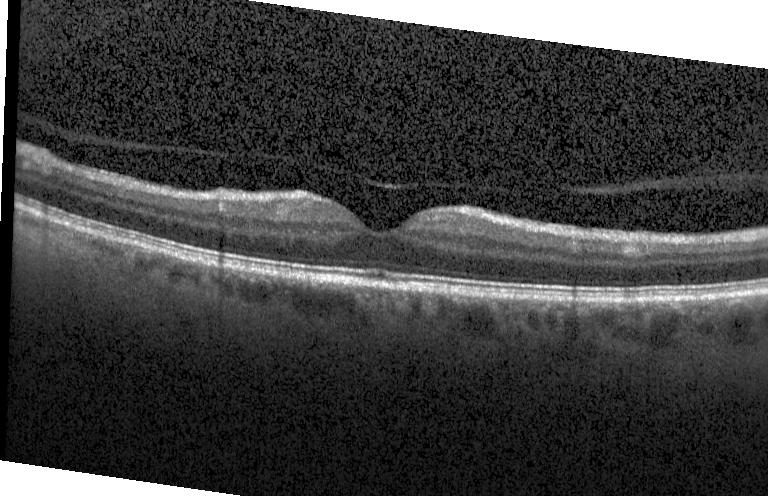 Optical coherence tomography scan — The scan shows no evidence of choroidal neovascularization, diabetic macular edema, or drusen.